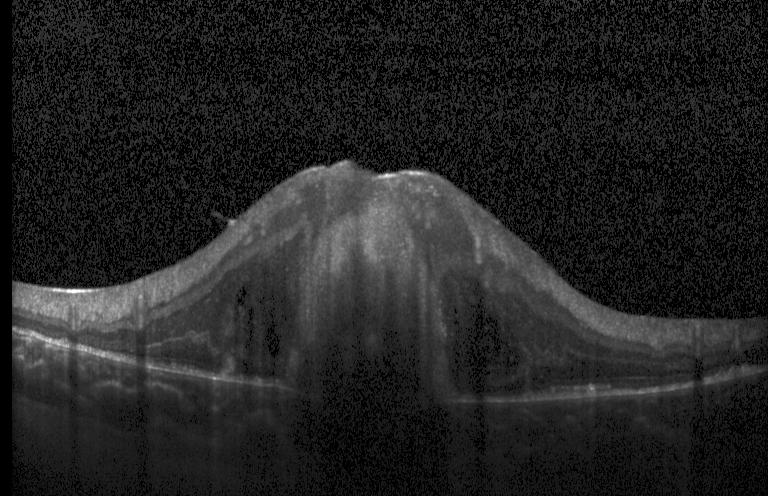

OCT B-scan; spectral-domain OCT; Heidelberg Spectralis — The scan shows a choroidal neovascular membrane.